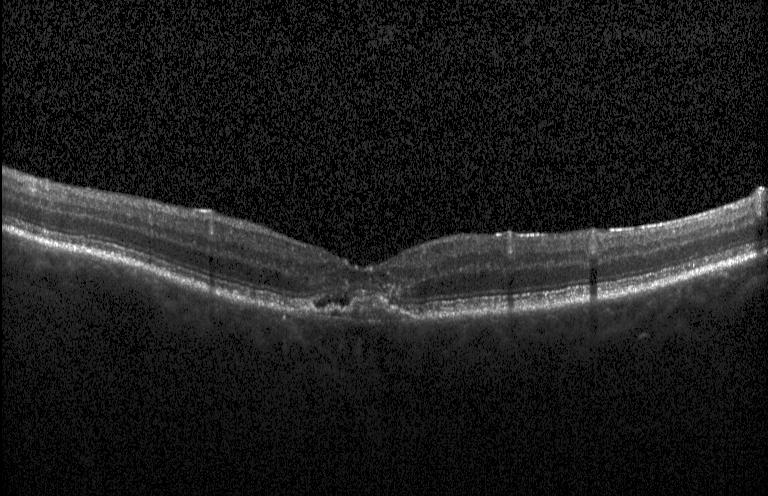 OCT line scan
Diagnosis: a choroidal neovascular membrane.